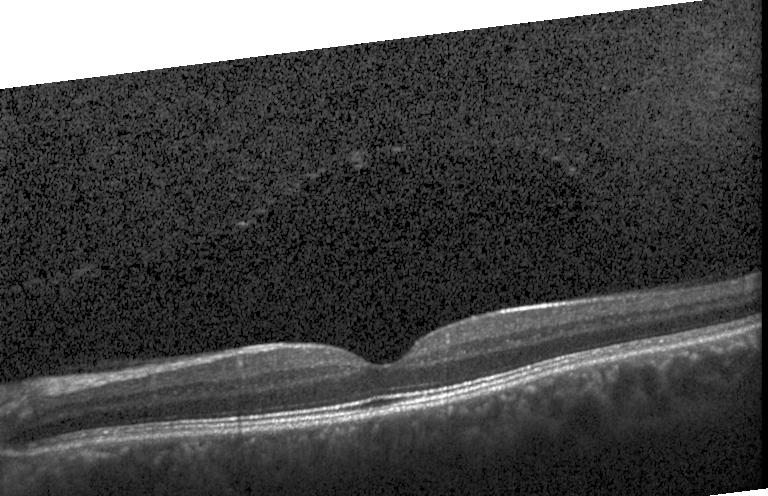
OCT B-scan
Finding: no evidence of choroidal neovascularization, diabetic macular edema, or drusen.